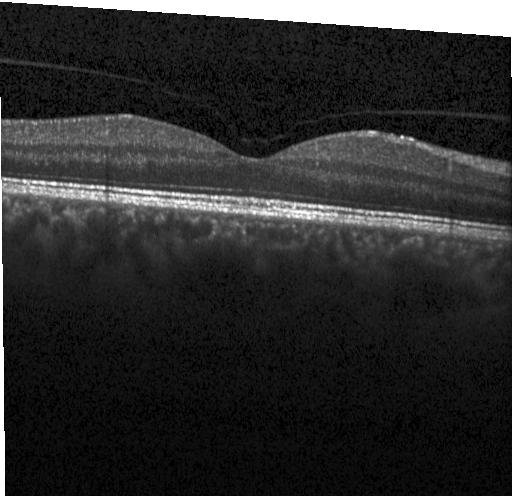
Centered on the fovea, Heidelberg Spectralis OCT system, optical coherence tomography scan — The scan shows no evidence of choroidal neovascularization, diabetic macular edema, or drusen.